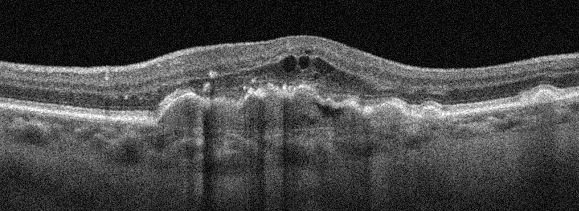
Optical coherence tomography scan. OS. Through the macula. Acquired on an Optovue Avanti RTVue XR — Dx: age-related macular degeneration.